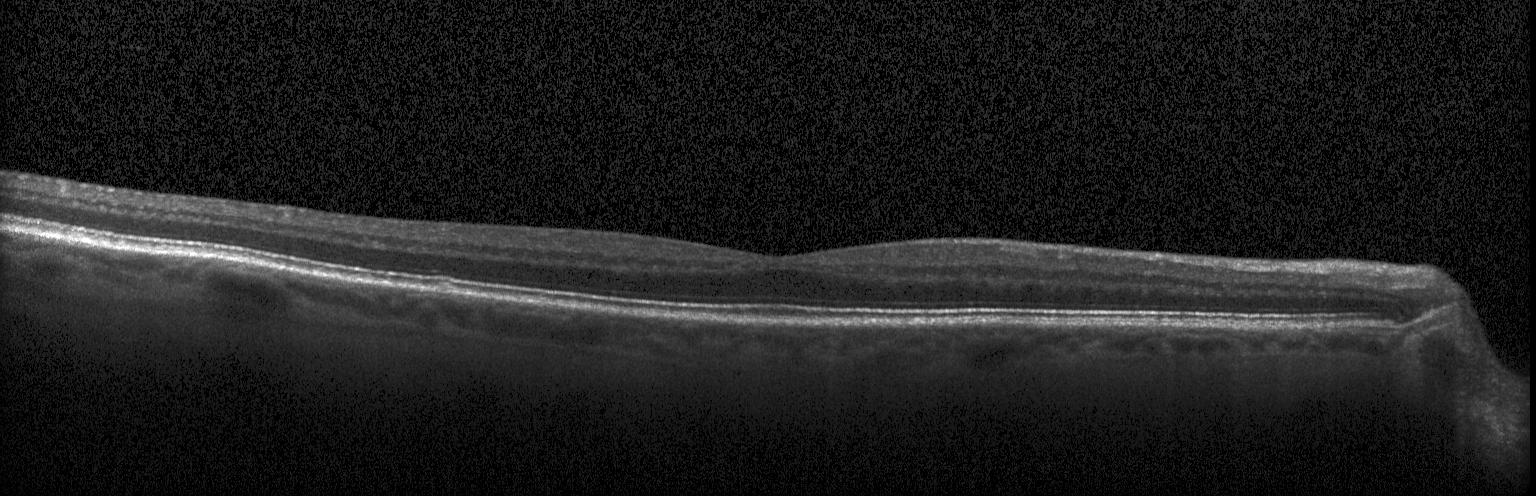
OCT B-scan · Heidelberg Spectralis · SD-OCT · through the macula. Diagnosis: no evidence of CNV, DME, or drusen.